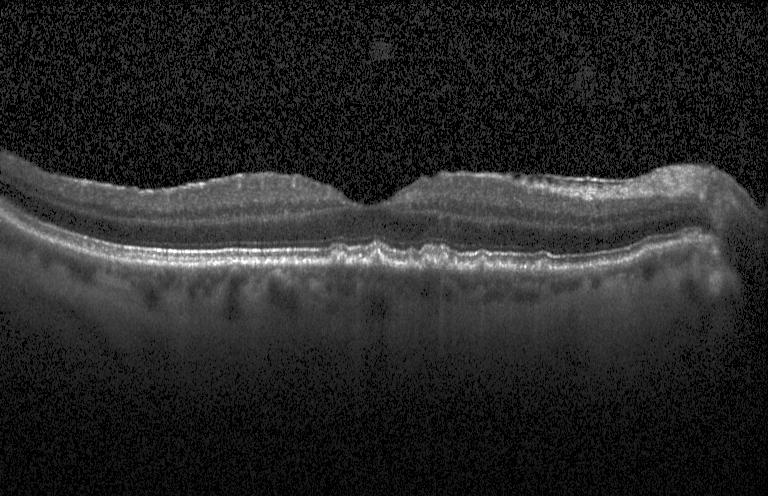 Impression: drusen.